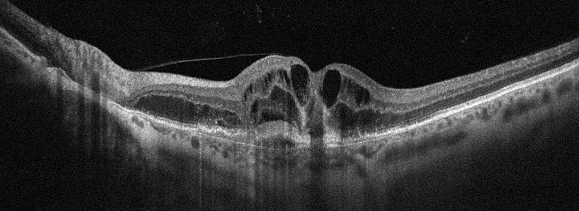 Oculus sinister. Fovea-centered. Optical coherence tomography B-scan. Instrument: Optovue Avanti RTVue XR — Impression: AMD.